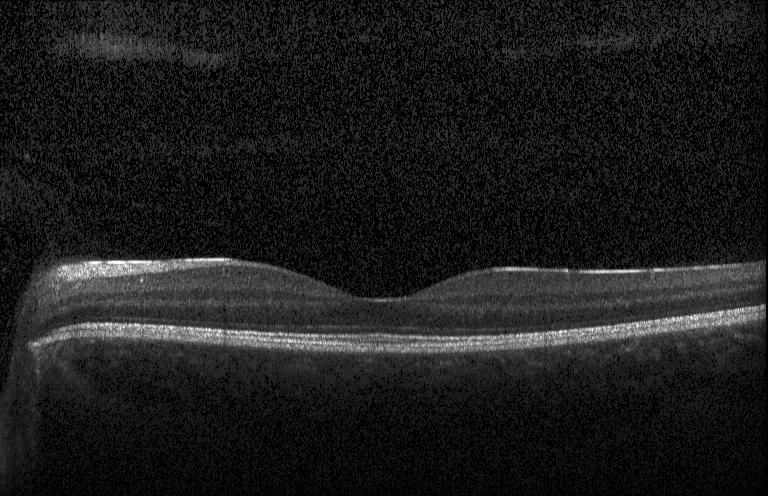

Retinal OCT cross-section
OCT finding: no evidence of choroidal neovascularization, diabetic macular edema, or drusen.